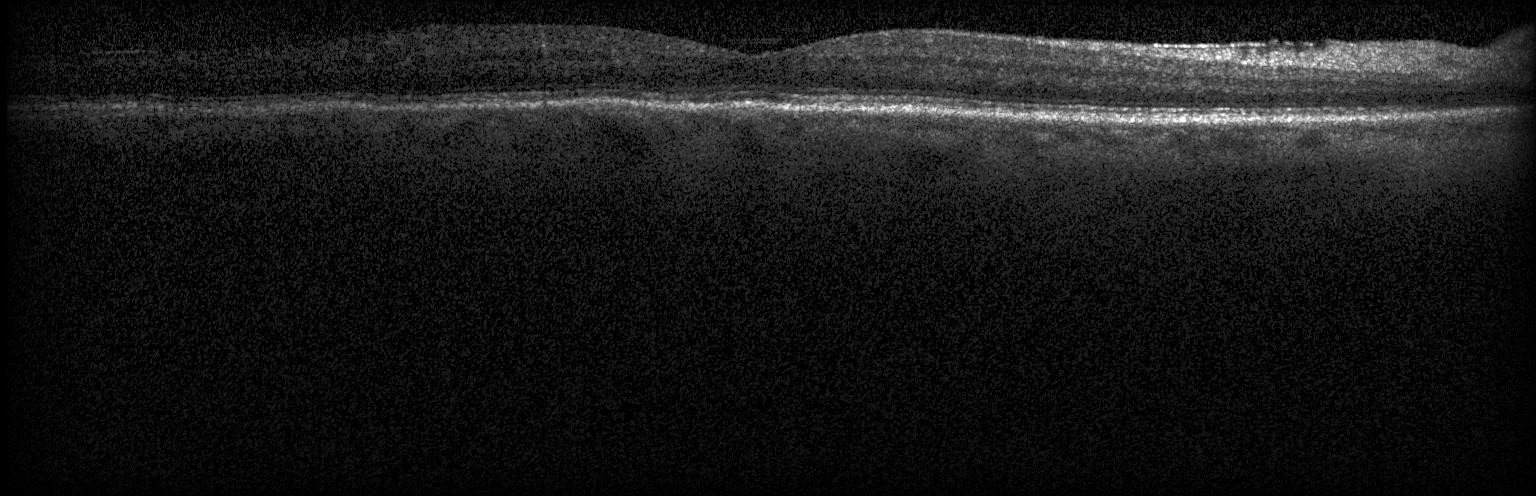

Optical coherence tomography B-scan · instrument: Heidelberg Spectralis — Diagnosis: no choroidal neovascularization, no diabetic macular edema, and no drusen.